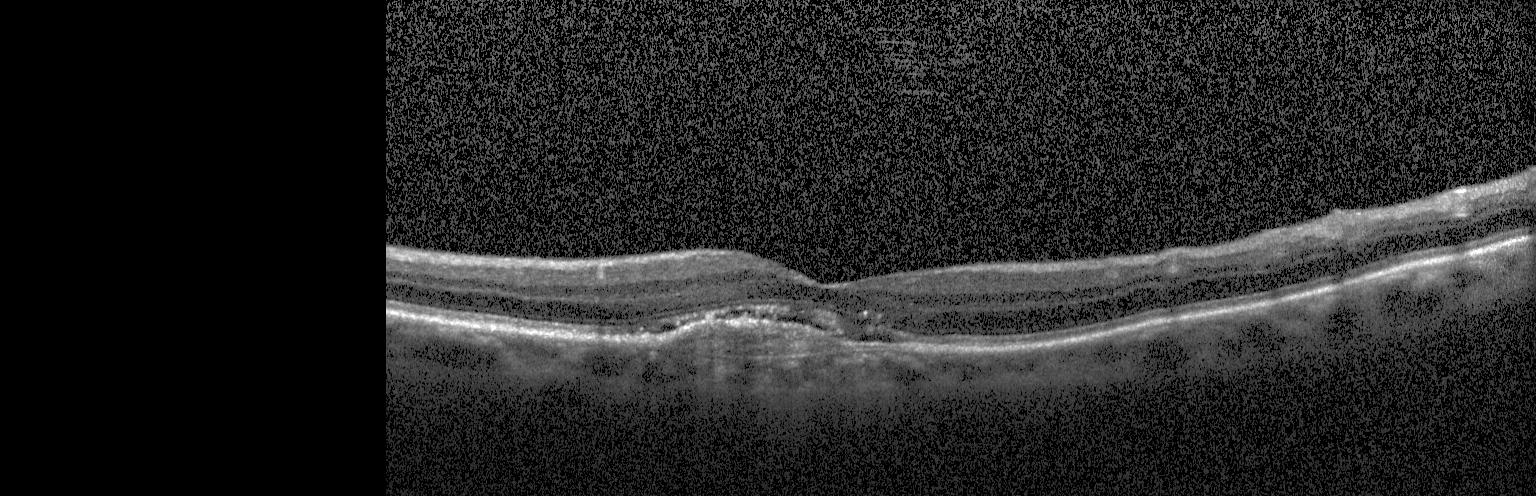

Instrument: Heidelberg Spectralis; retinal OCT B-scan.
OCT finding: a choroidal neovascular membrane.